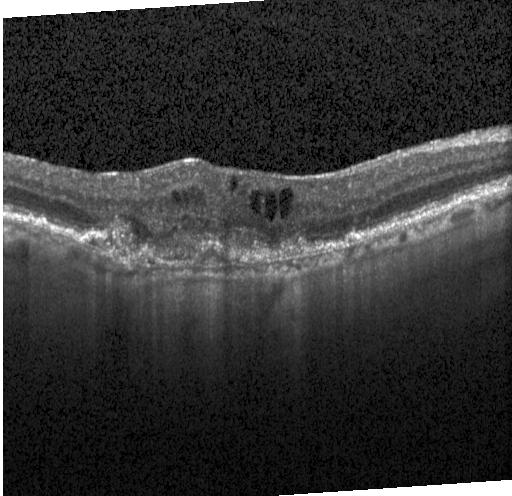

Impression: choroidal neovascularization (CNV).